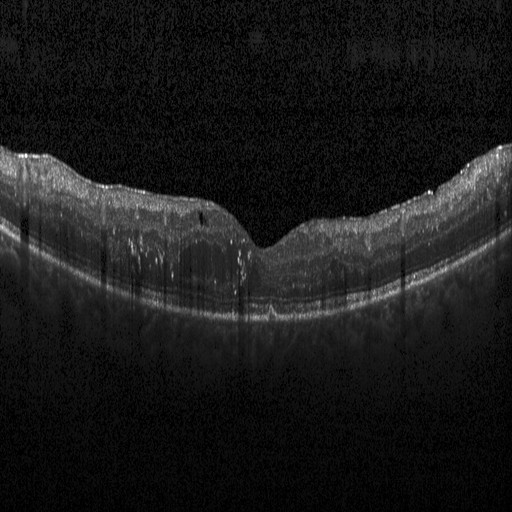 Spectral-domain optical coherence tomography, through the macula, acquired on a Heidelberg Spectralis, OCT B-scan. Diabetic macular edema.